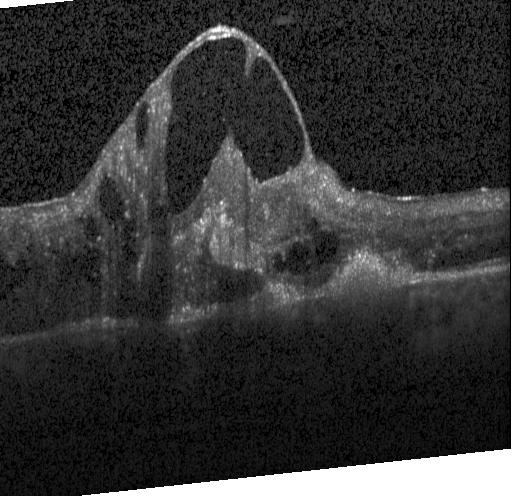
Through the macula, OCT B-scan.
Assessment: choroidal neovascularization (CNV).